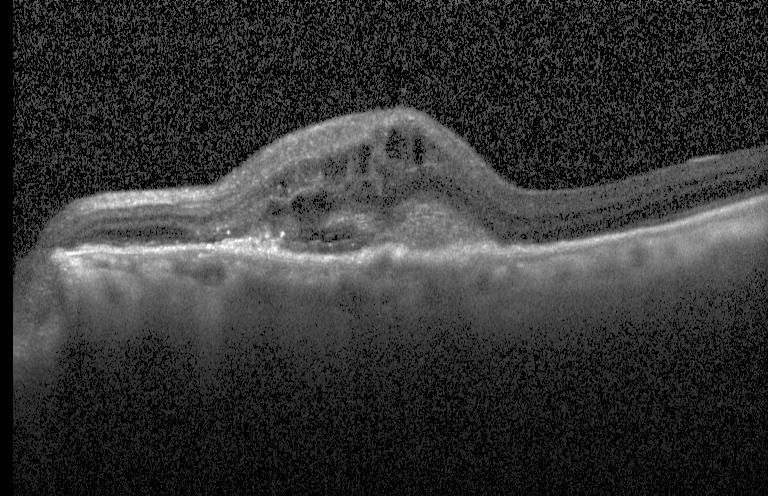 Retinal OCT cross-section; instrument: Heidelberg Spectralis.
This B-scan demonstrates choroidal neovascularization.